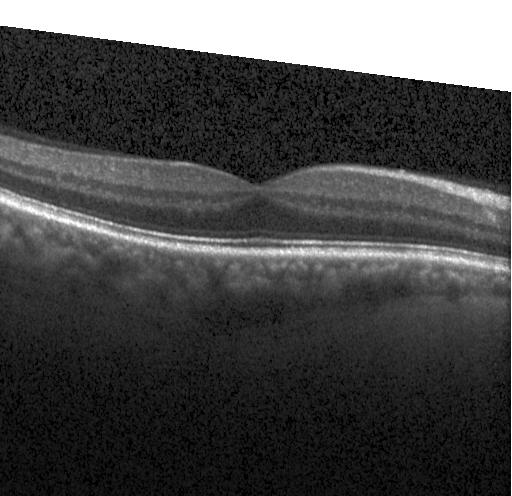
Impression: no evidence of choroidal neovascularization, diabetic macular edema, or drusen.